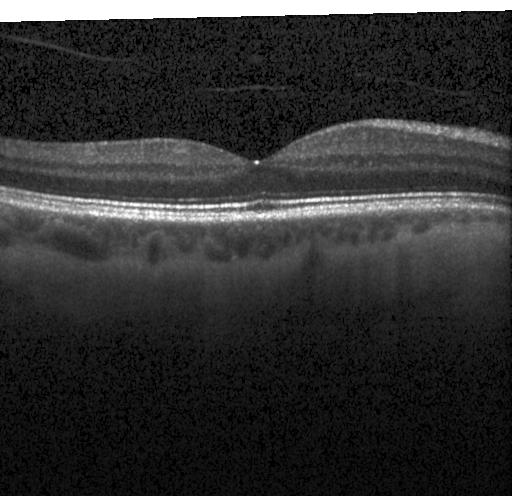

SD-OCT; retinal OCT cross-section
Impression: no choroidal neovascularization, diabetic macular edema, or drusen.